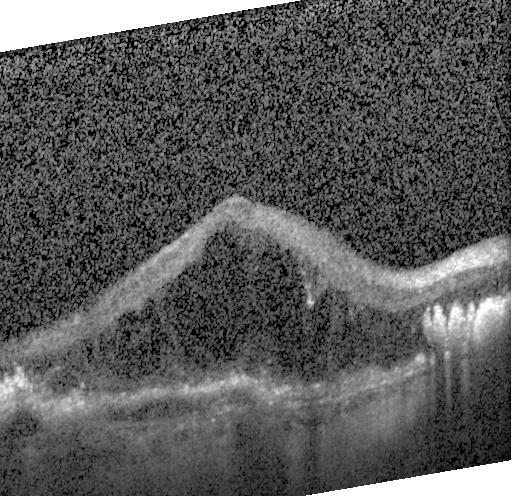

Spectral-domain OCT B-scan: CNV.